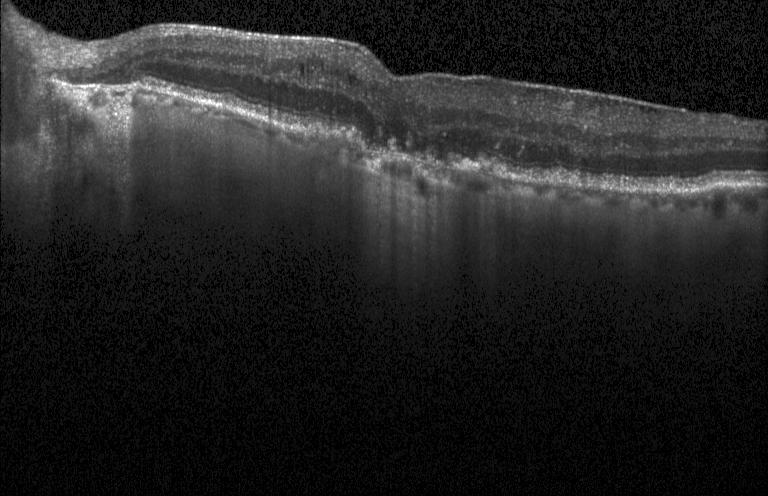 Spectral-domain OCT, instrument: Heidelberg Spectralis, macular scan, OCT B-scan — This B-scan demonstrates a choroidal neovascular membrane.